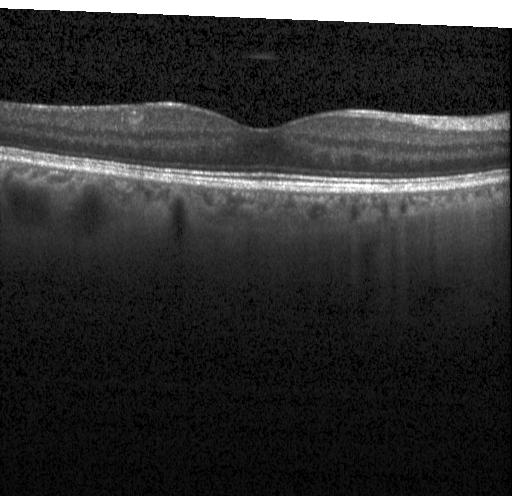 Spectral-domain OCT · optical coherence tomography B-scan · centered on the fovea · Heidelberg Spectralis
Macular OCT: no choroidal neovascularization, no diabetic macular edema, and no drusen.